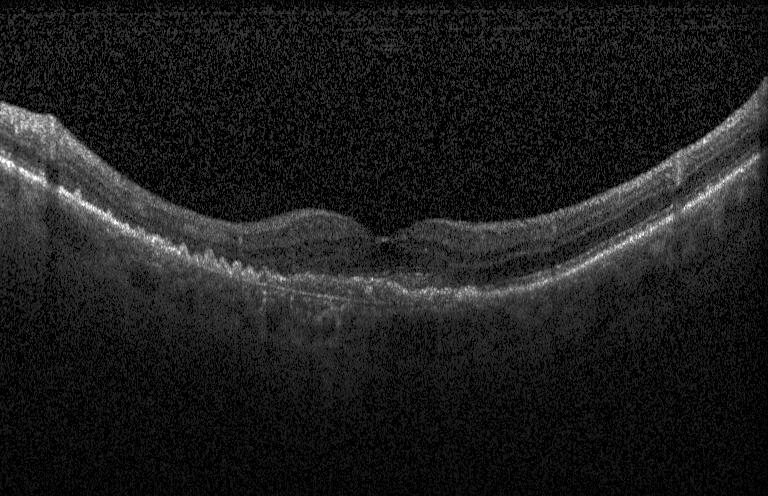
Macular scan, instrument: Heidelberg Spectralis, spectral-domain OCT, retinal OCT cross-section. Diagnosis: a choroidal neovascular membrane.